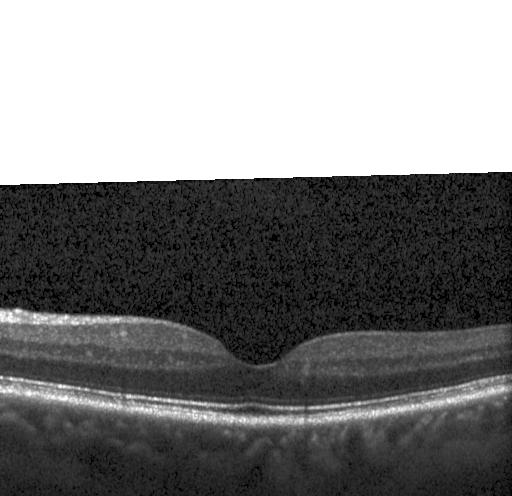
Macular OCT: no choroidal neovascularization, no diabetic macular edema, and no drusen.